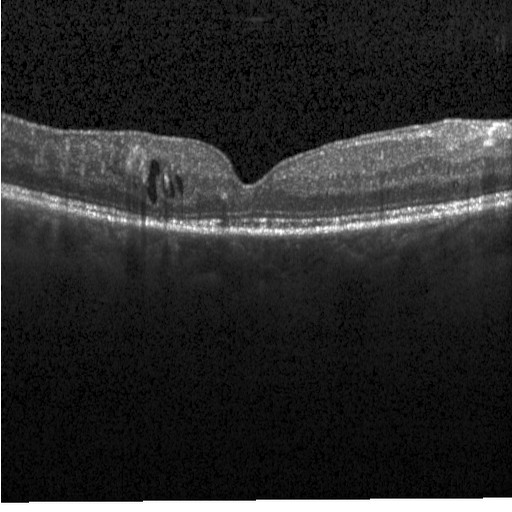

Retinal OCT cross-section; instrument: Heidelberg Spectralis; spectral-domain OCT — Diabetic macular edema (DME).